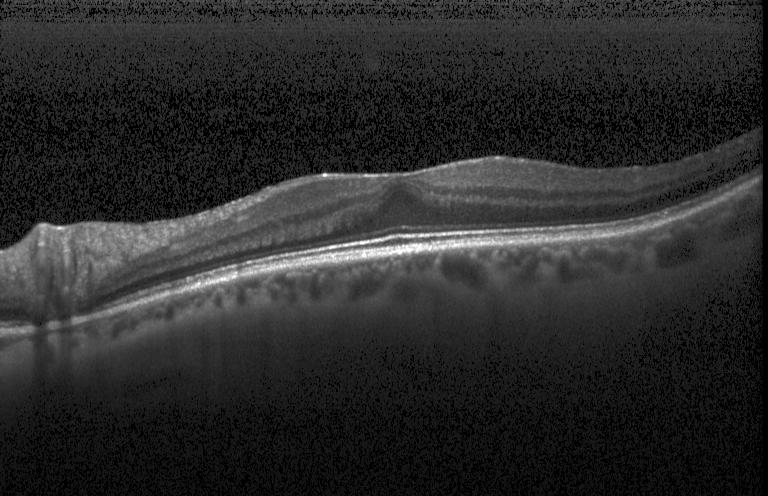
OCT B-scan · SD-OCT.
No choroidal neovascularization, no diabetic macular edema, and no drusen.